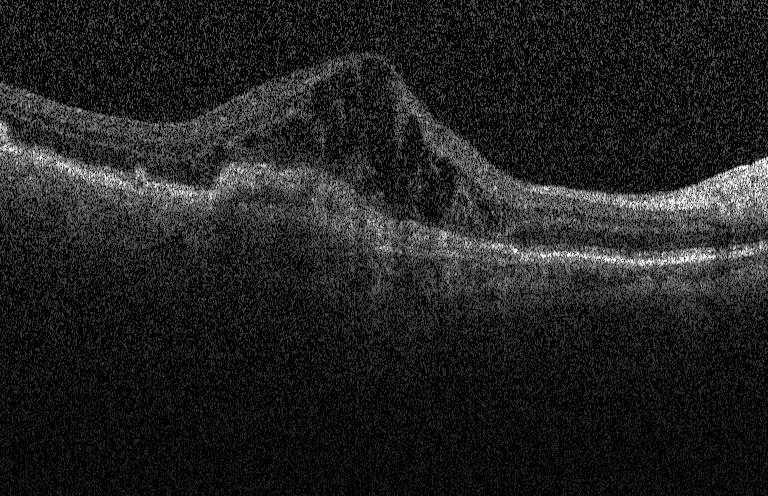
Diagnosis: choroidal neovascularization (CNV).